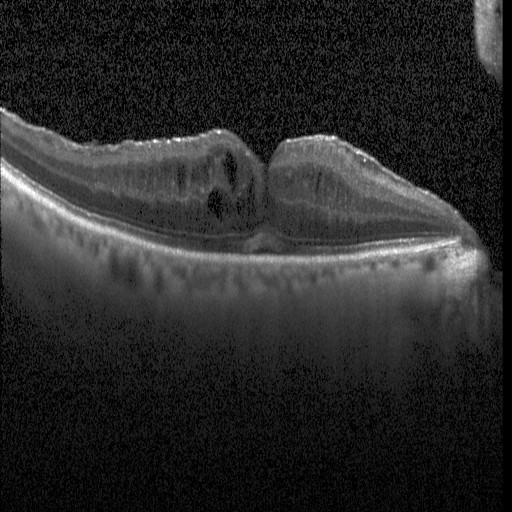

Dx: diabetic macular edema (DME).